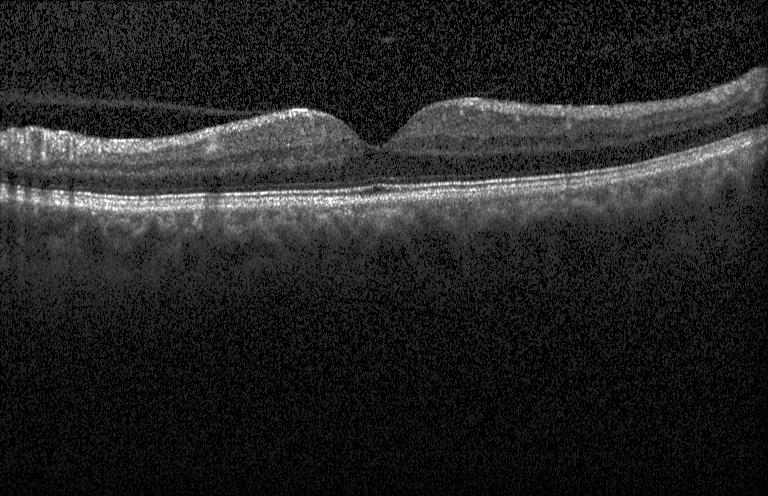 The scan shows no CNV, no DME, and no drusen.